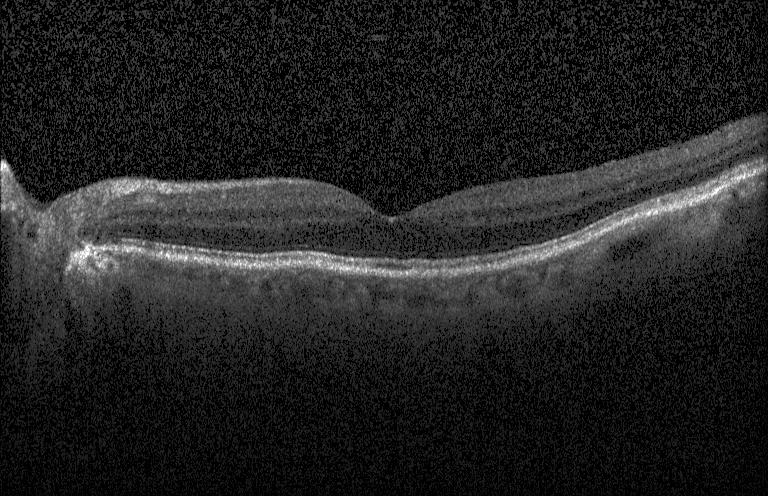 Retinal OCT cross-section; spectral-domain OCT
Finding: no evidence of choroidal neovascularization, diabetic macular edema, or drusen.